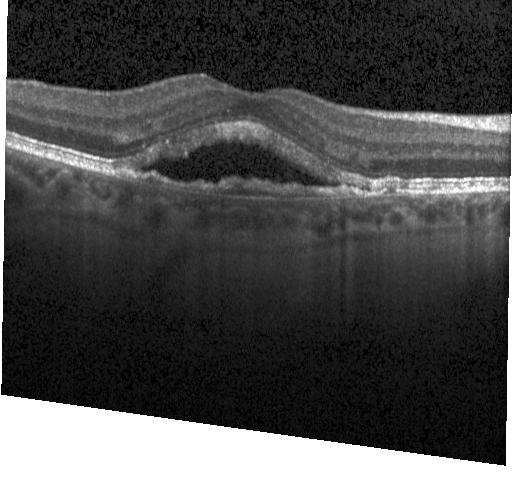
Dx: a choroidal neovascular membrane.